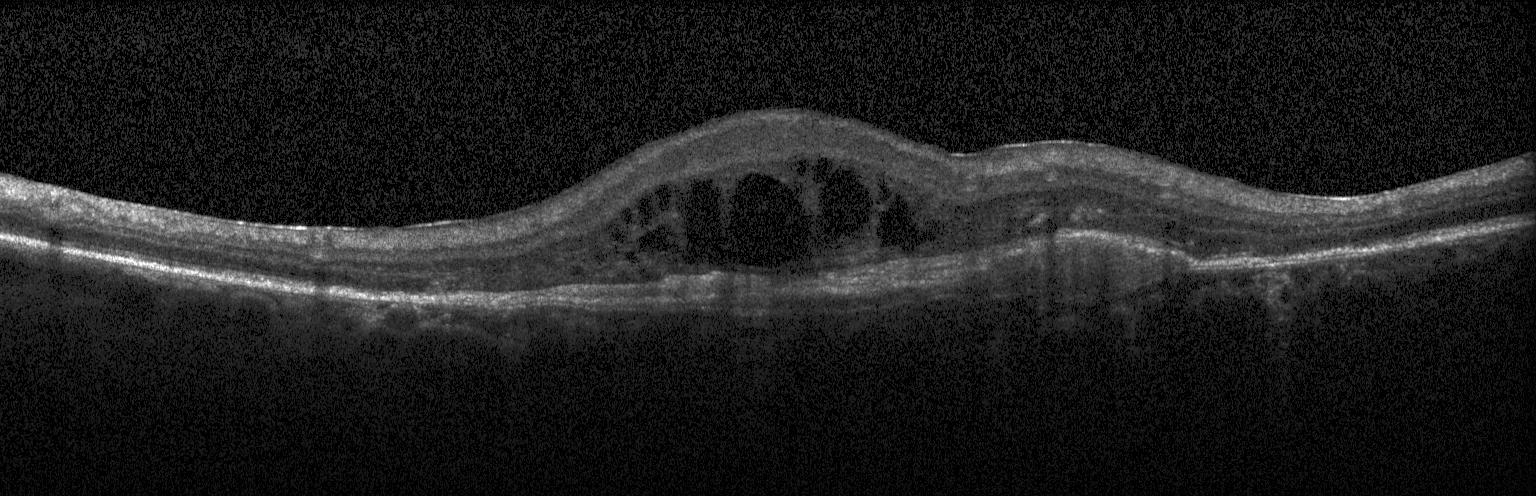

OCT finding: choroidal neovascularization.